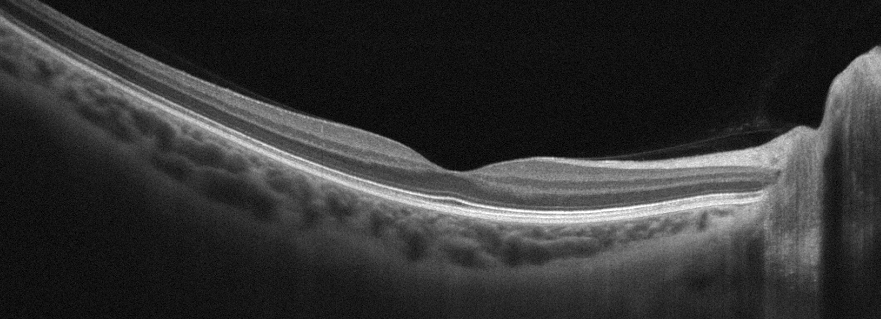 Through the macula · retinal OCT B-scan. Dx: no AMD, DME, ERM, RAO, RVO, or VID.